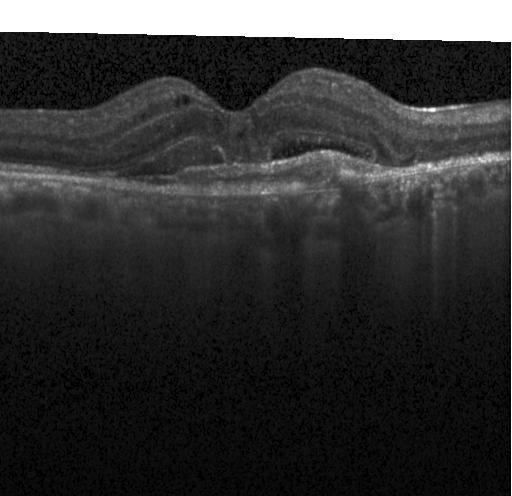

Macular OCT demonstrating choroidal neovascularization.